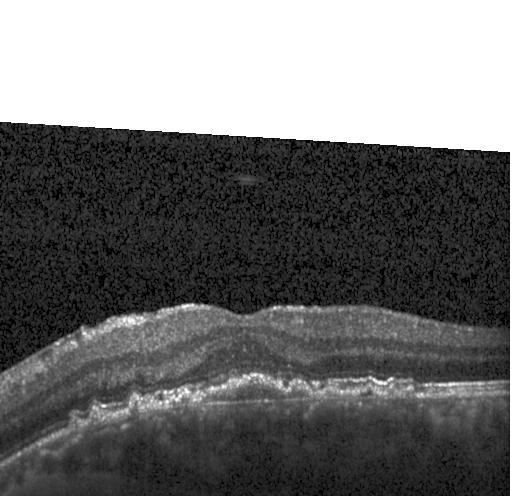

Retinal OCT B-scan.
The scan shows CNV.